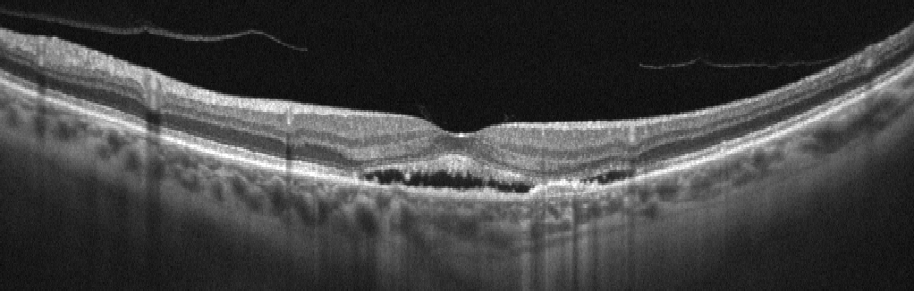 Assessment: AMD.